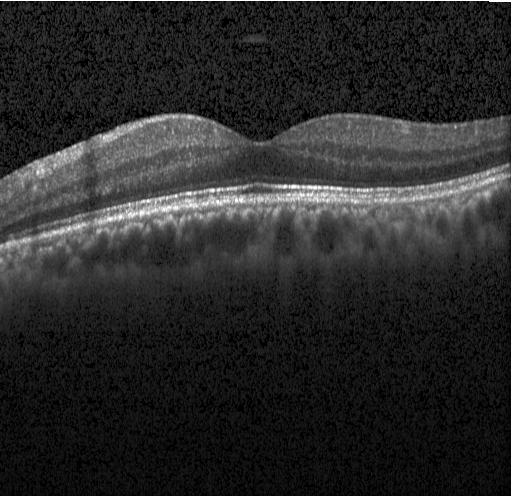 Optical coherence tomography B-scan · spectral-domain optical coherence tomography · macular scan — Diagnosis: no evidence of choroidal neovascularization, diabetic macular edema, or drusen.